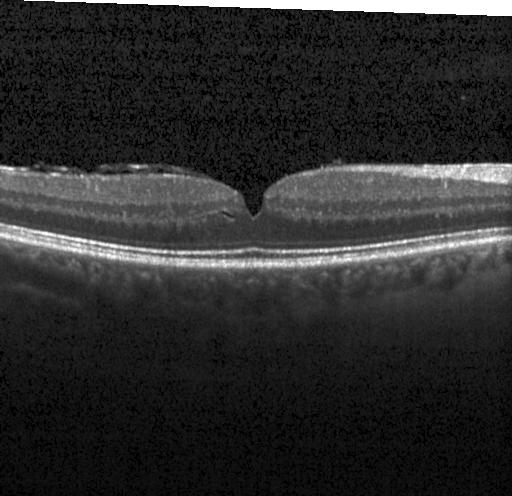 Acquired on a Heidelberg Spectralis · retinal OCT B-scan · through the macula · spectral-domain OCT. Finding: DME.